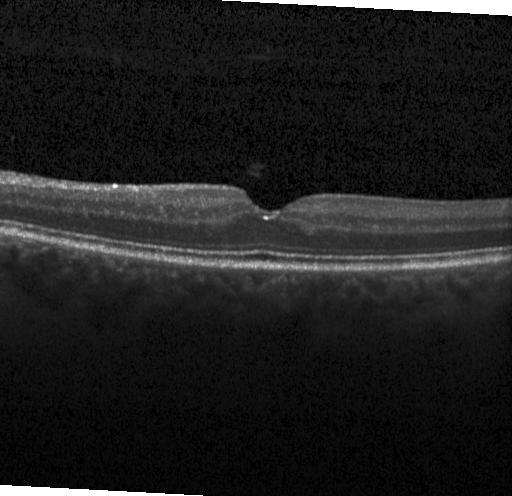 Retinal OCT B-scan.
Finding: no evidence of choroidal neovascularization, diabetic macular edema, or drusen.